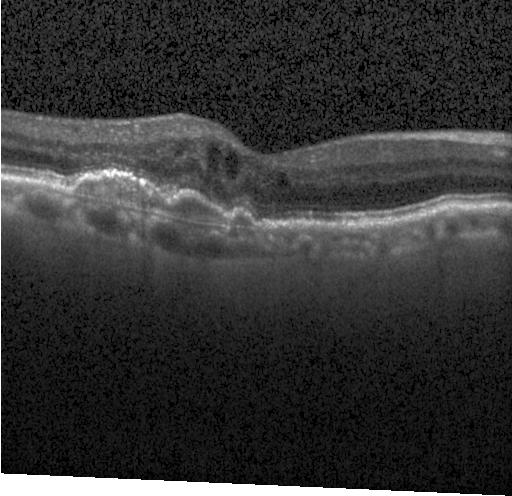

Horizontal scan through the fovea; retinal OCT B-scan. CNV.